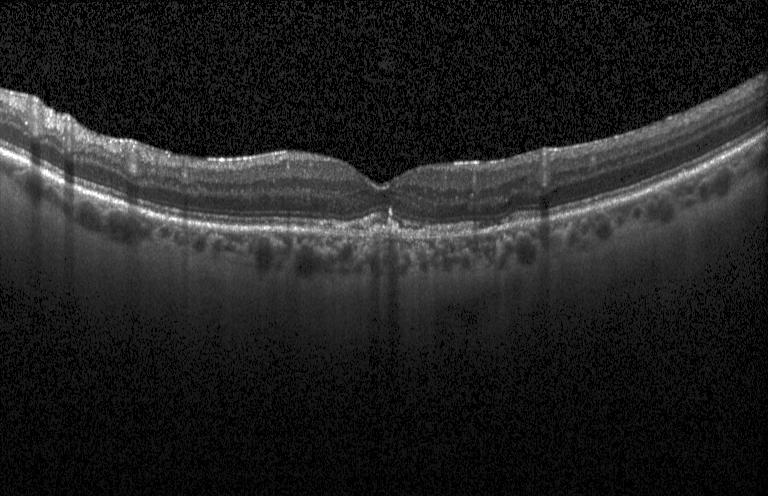 Finding: CNV.